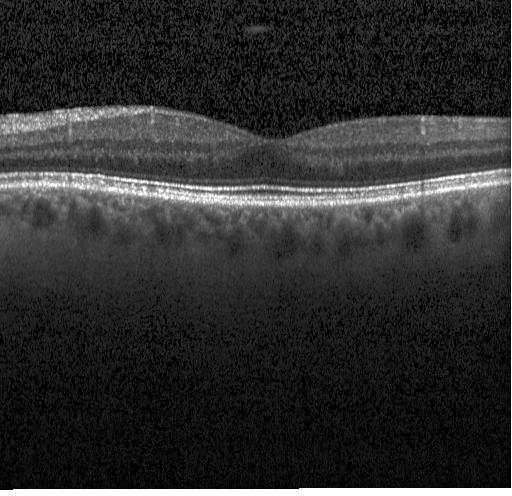
Retinal OCT B-scan
Diagnosis: no evidence of CNV, DME, or drusen.